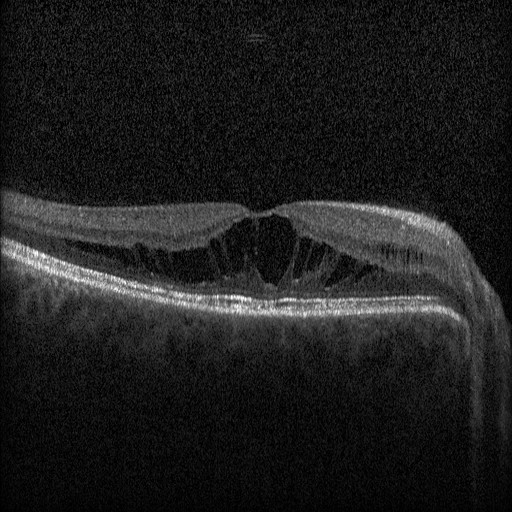
Finding: diabetic macular edema (DME).